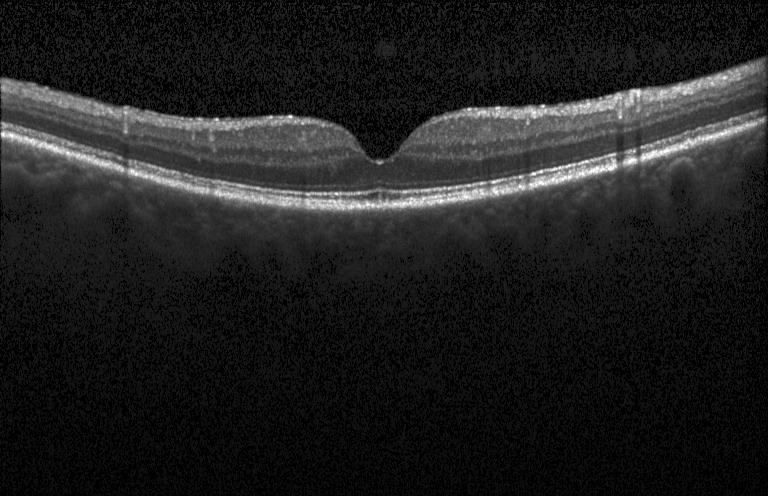 Retinal OCT cross-section showing no choroidal neovascularization, no diabetic macular edema, and no drusen.